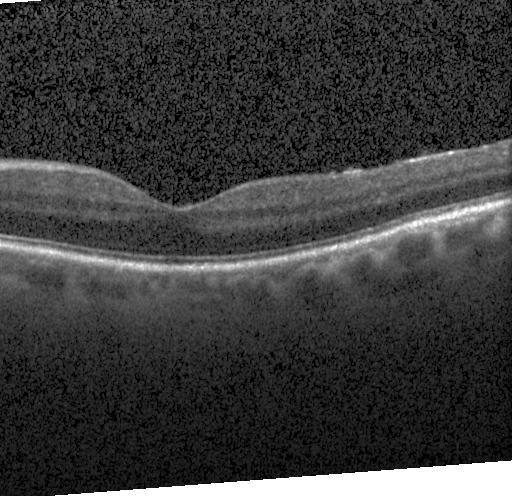
OCT B-scan showing neither choroidal neovascularization, diabetic macular edema, nor drusen.